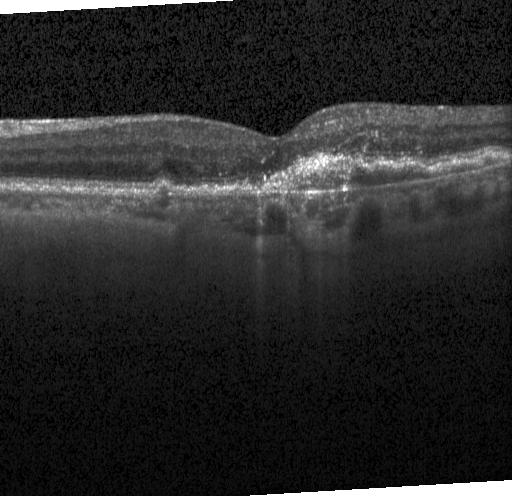 Finding: a choroidal neovascular membrane.